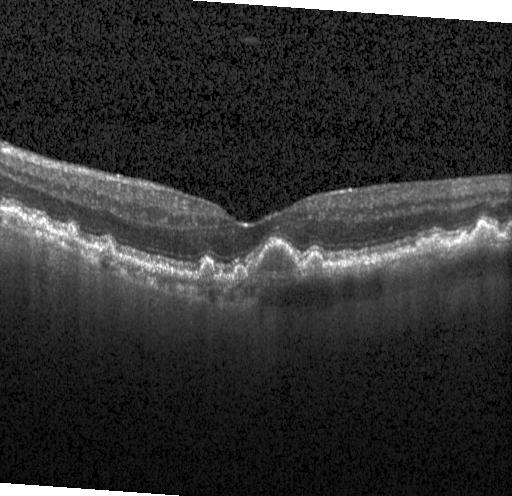
This B-scan demonstrates multiple drusen.